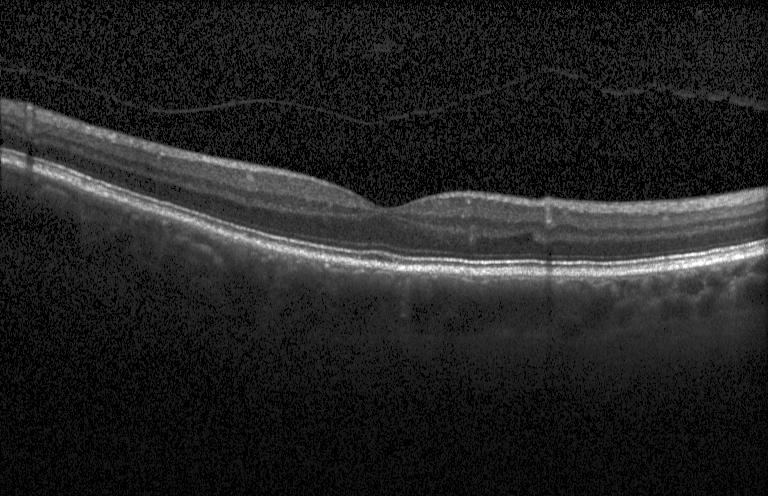 Spectral-domain OCT · OCT B-scan.
Diagnosis: no choroidal neovascularization, no diabetic macular edema, and no drusen.